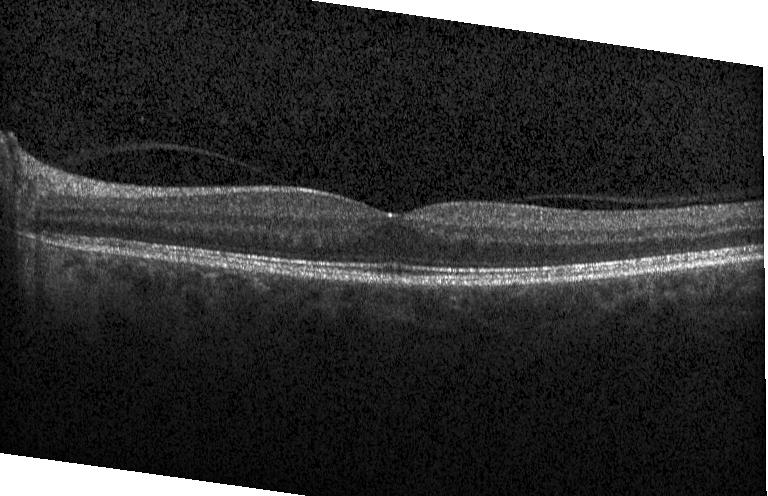

Diagnosis: neither CNV, DME, nor drusen.